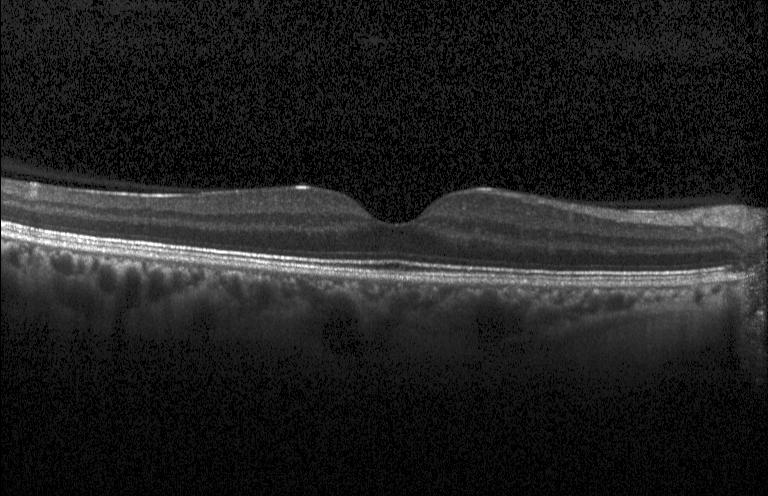
Heidelberg Spectralis OCT system. Optical coherence tomography scan — This B-scan demonstrates no evidence of choroidal neovascularization, diabetic macular edema, or drusen.